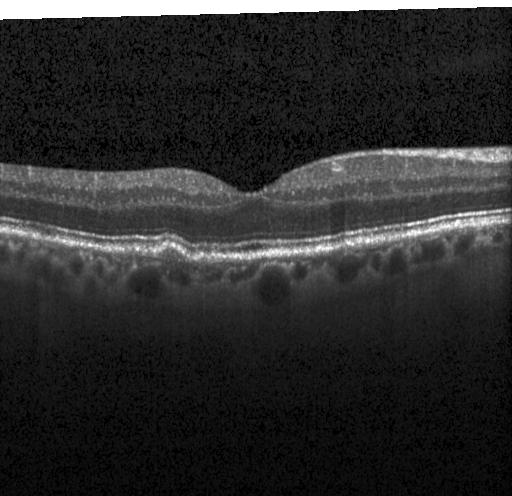
Optical coherence tomography scan · instrument: Heidelberg Spectralis.
Impression: drusen.